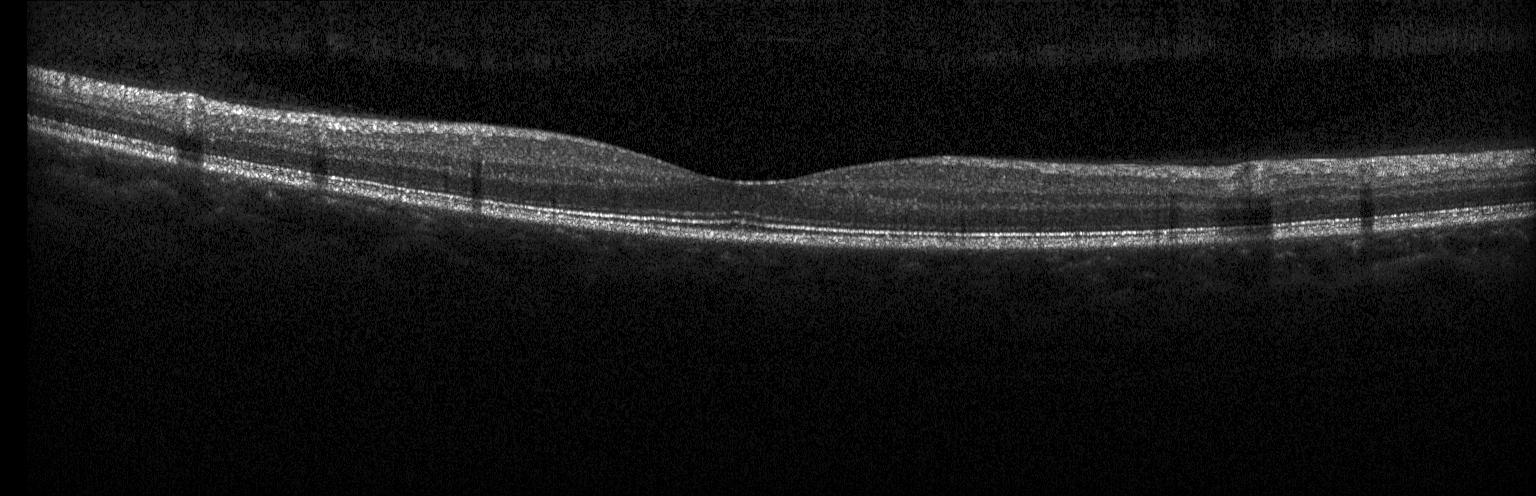

Diagnosis: no evidence of choroidal neovascularization, diabetic macular edema, or drusen.